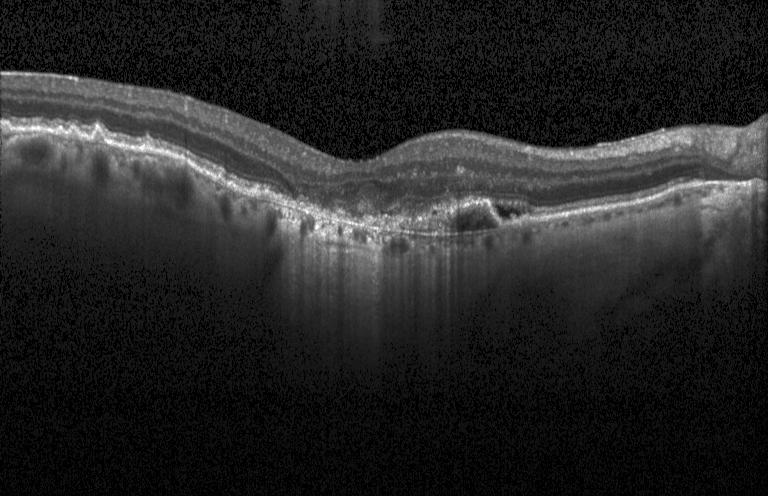
Retinal OCT cross-section · Heidelberg Spectralis · horizontal scan through the fovea. Finding: a choroidal neovascular membrane.